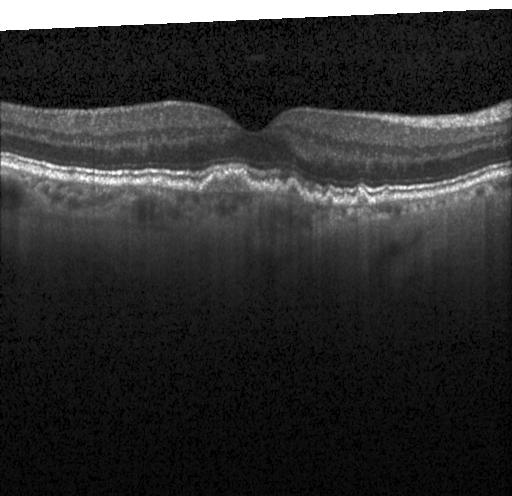

Optical coherence tomography B-scan — Diagnosis: sub-RPE drusenoid deposits.